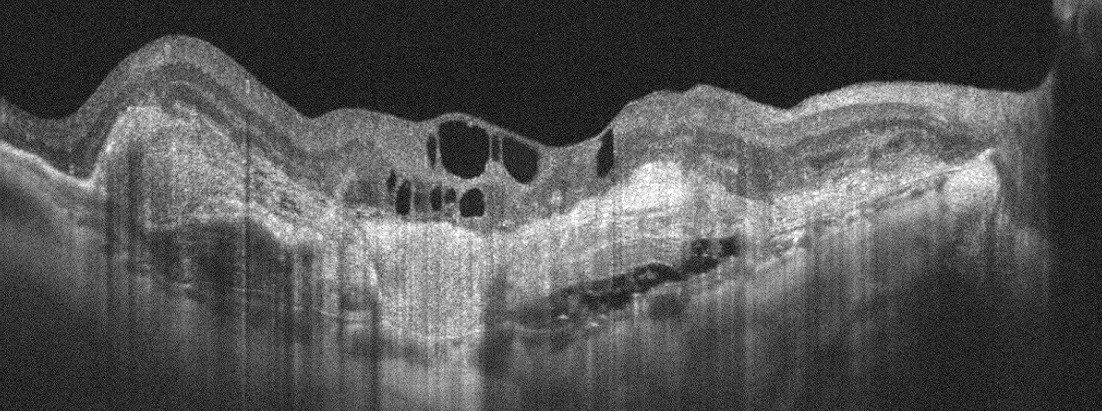 OCT scan showing AMD.